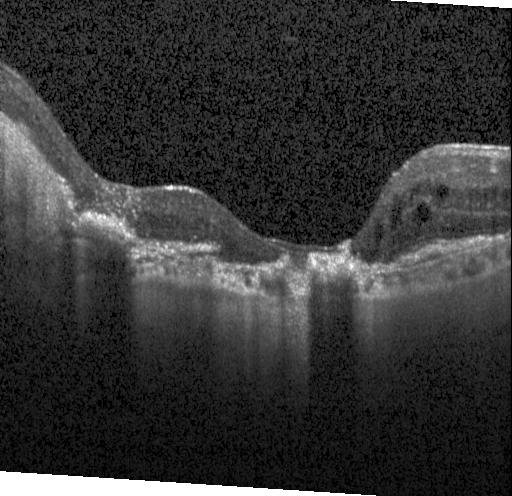
OCT B-scan · SD-OCT.
The scan shows CNV.